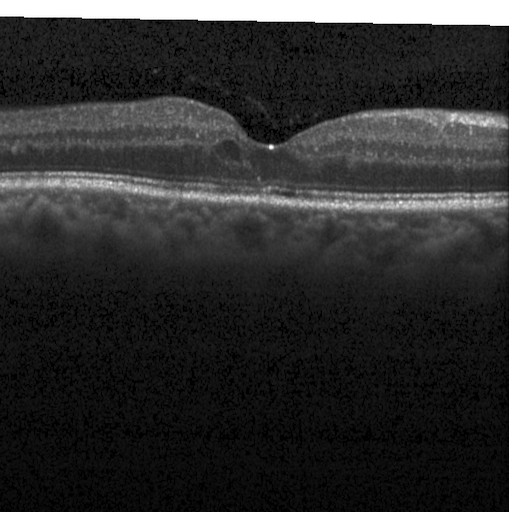
Acquired on a Heidelberg Spectralis, retinal OCT cross-section
DME.